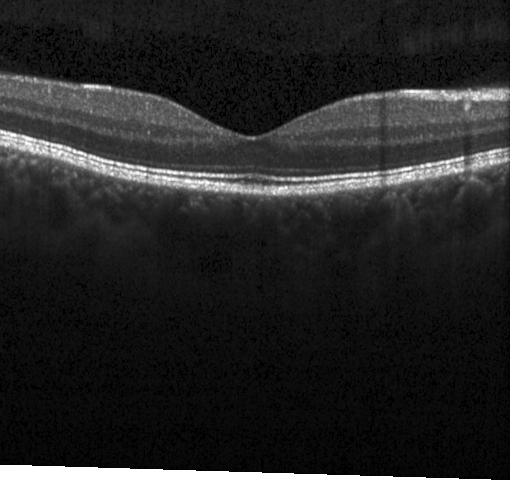
Diagnosis: no CNV, no DME, and no drusen.